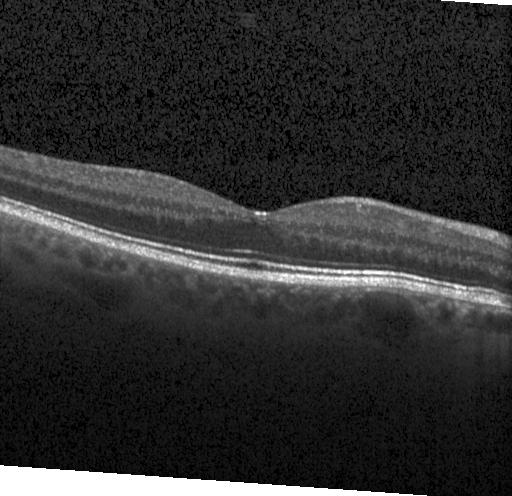 SD-OCT, Heidelberg Spectralis, macular scan, retinal OCT B-scan. This B-scan demonstrates no evidence of choroidal neovascularization, diabetic macular edema, or drusen.